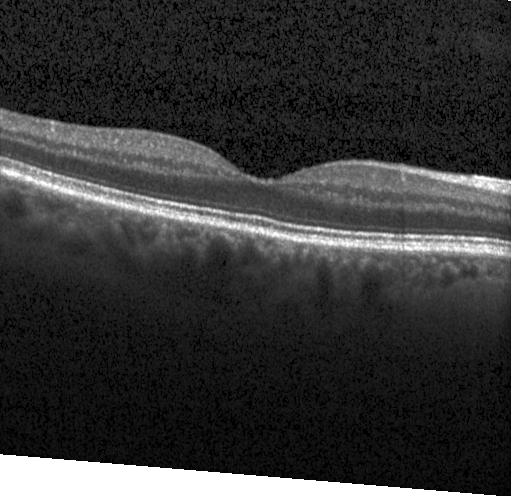
OCT line scan, acquired on a Heidelberg Spectralis — OCT finding: neither choroidal neovascularization, diabetic macular edema, nor drusen.